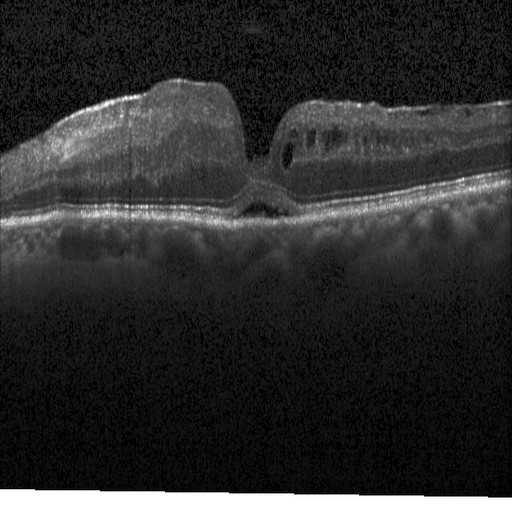
Retinal OCT cross-section — Finding: diabetic macular edema (DME).